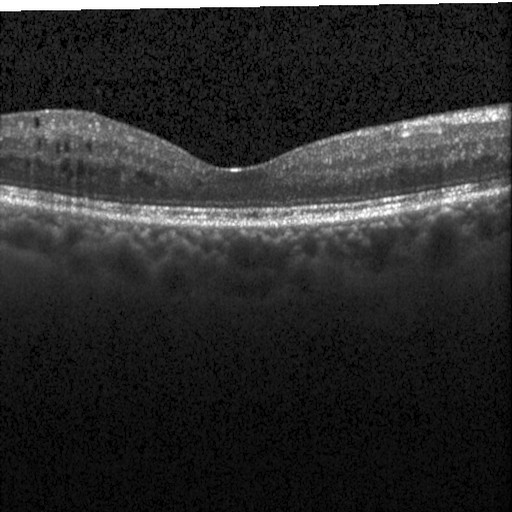 Instrument: Heidelberg Spectralis, OCT B-scan, macular scan, spectral-domain OCT. The scan shows diabetic macular edema (DME).